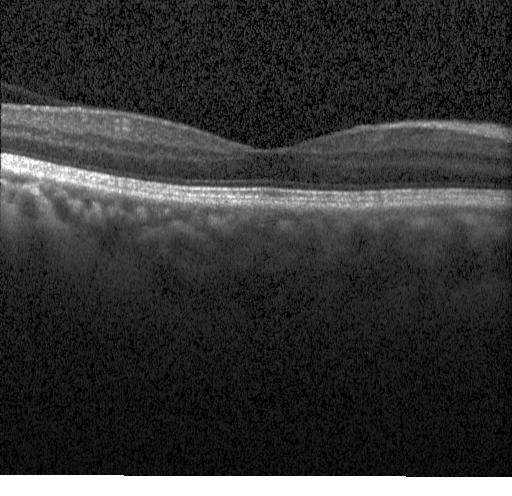 Macular OCT: neither choroidal neovascularization, diabetic macular edema, nor drusen.